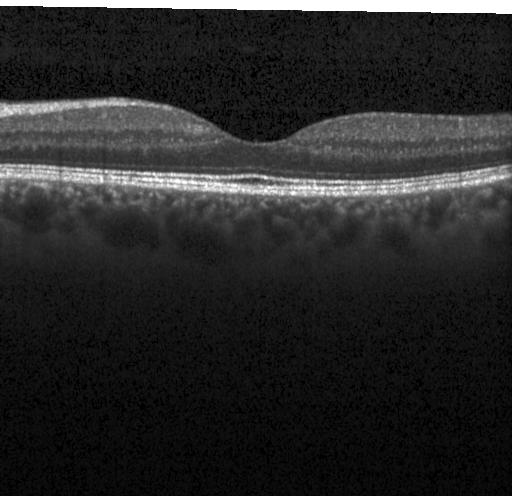
Diagnosis: neither choroidal neovascularization, diabetic macular edema, nor drusen.